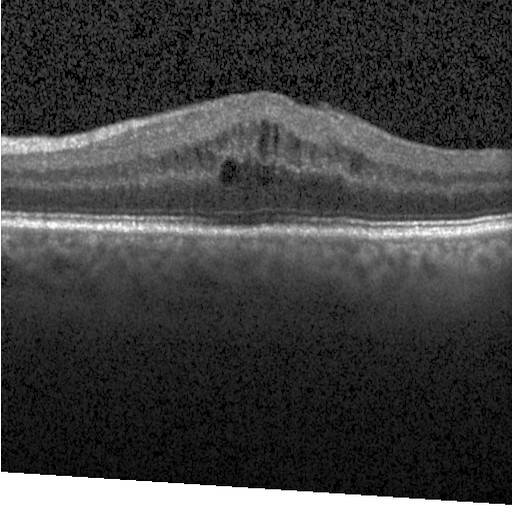
Optical coherence tomography scan. Diagnosis: diabetic macular edema.